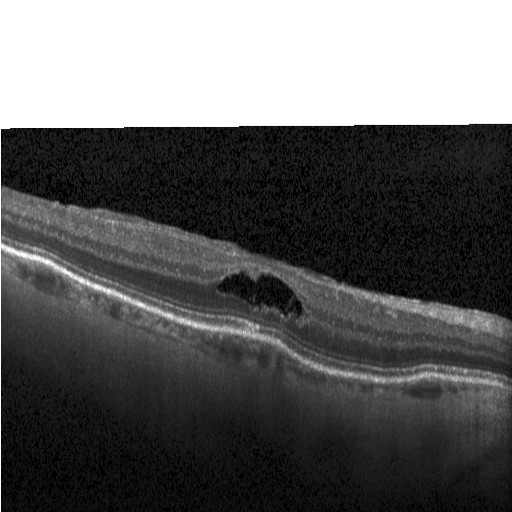 Optical coherence tomography B-scan — Finding: diabetic macular edema.